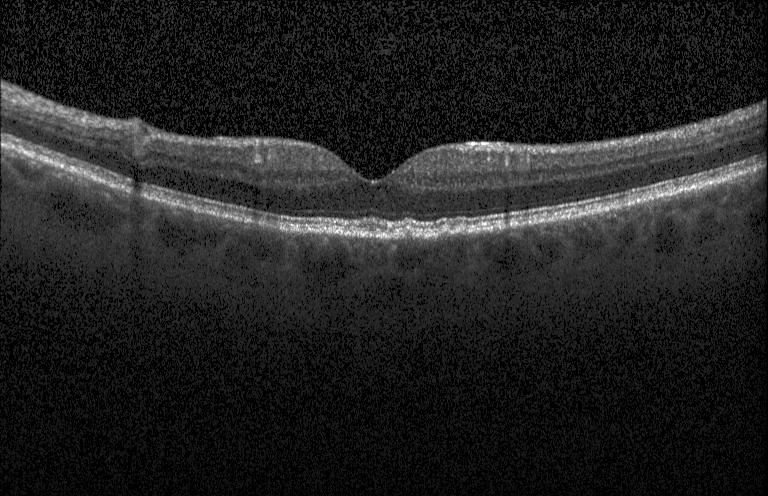 Retinal OCT cross-section — Finding: sub-RPE drusenoid deposits.